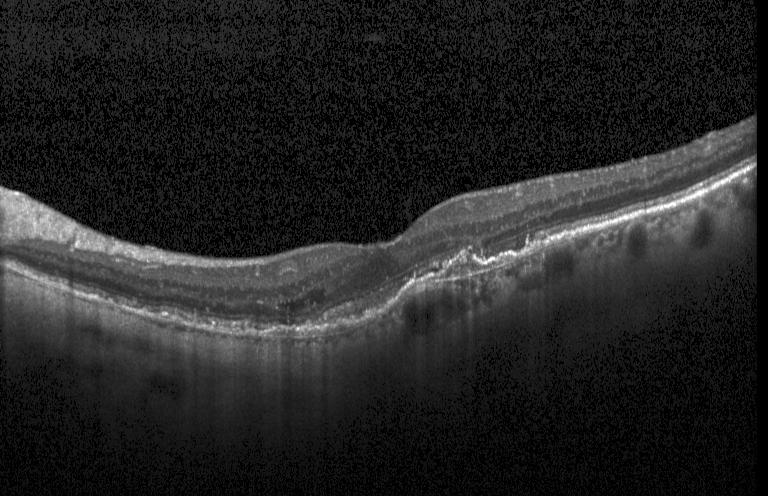 Retinal OCT cross-section; macular scan; Heidelberg Spectralis OCT system
The scan shows choroidal neovascularization.